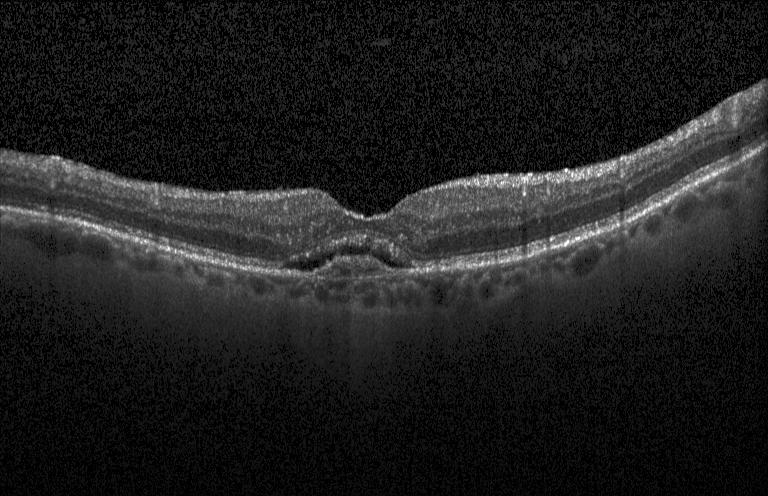
Optical coherence tomography B-scan, Heidelberg Spectralis.
A choroidal neovascular membrane.